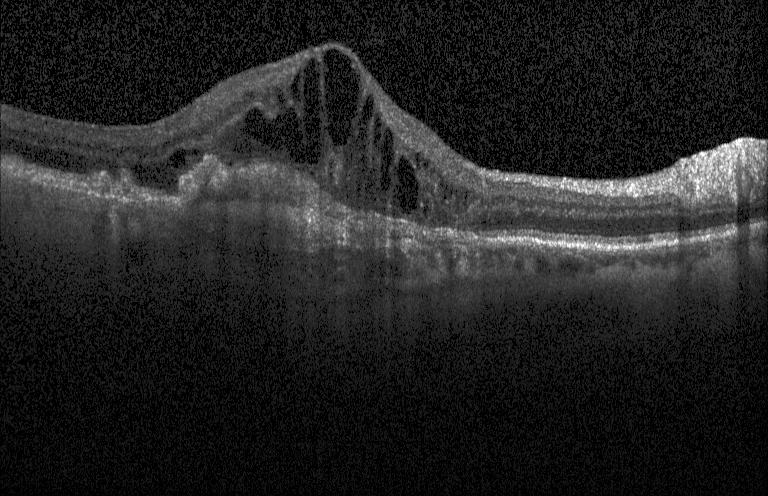 SD-OCT. OCT B-scan. Macular scan
Diagnosis: CNV.